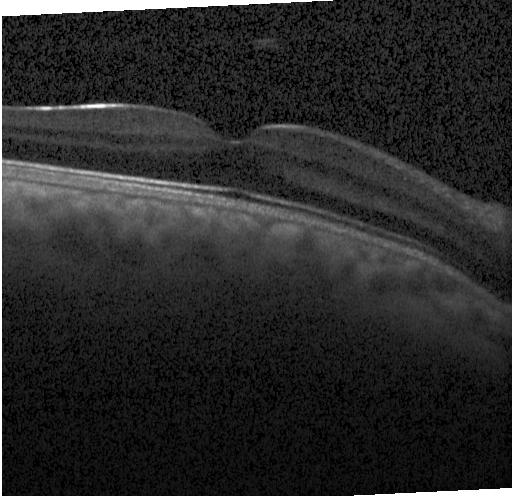
Spectral-domain OCT; retinal OCT B-scan; macular scan. Finding: no choroidal neovascularization, no diabetic macular edema, and no drusen.